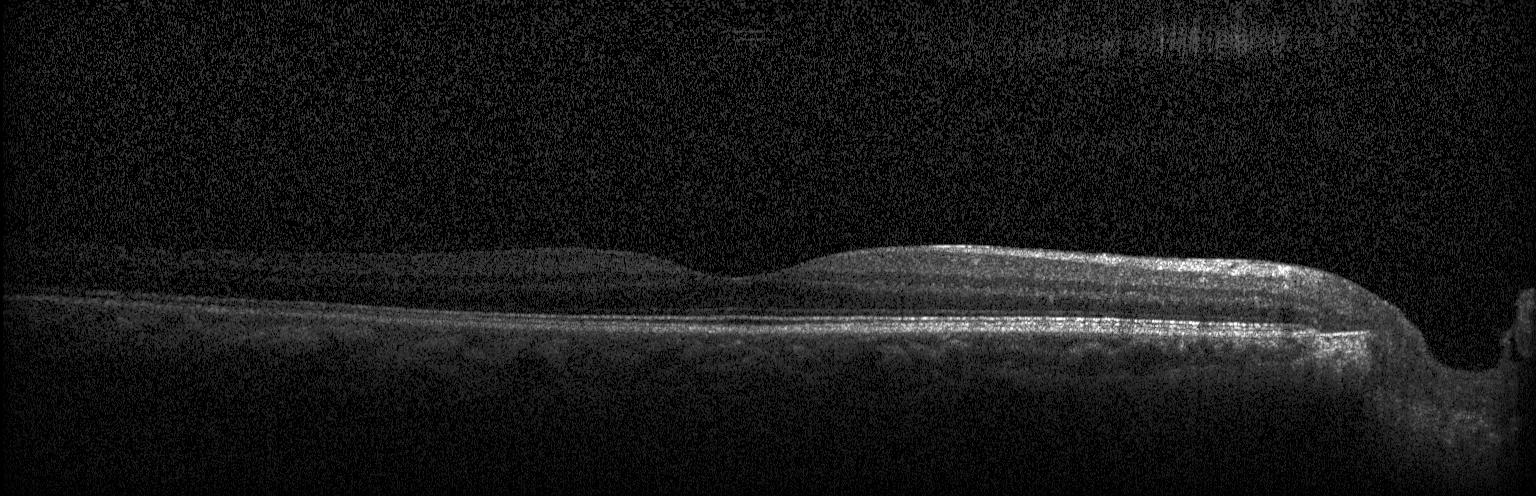
Impression: no evidence of choroidal neovascularization, diabetic macular edema, or drusen.